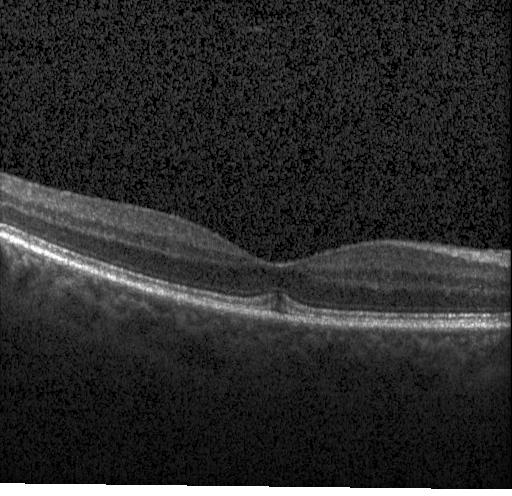
OCT B-scan. OCT finding: neither choroidal neovascularization, diabetic macular edema, nor drusen.